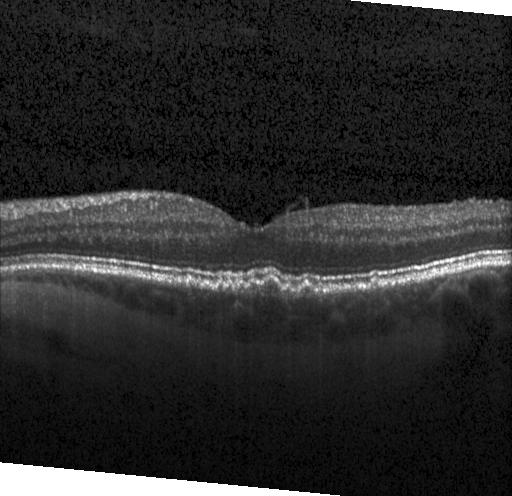
Retinal OCT cross-section. SD-OCT. Through the macula
OCT finding: sub-RPE drusenoid deposits.